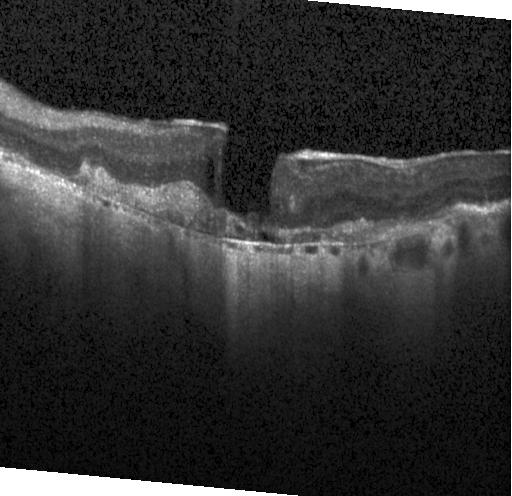

Fovea-centered. Retinal OCT cross-section
Choroidal neovascularization.